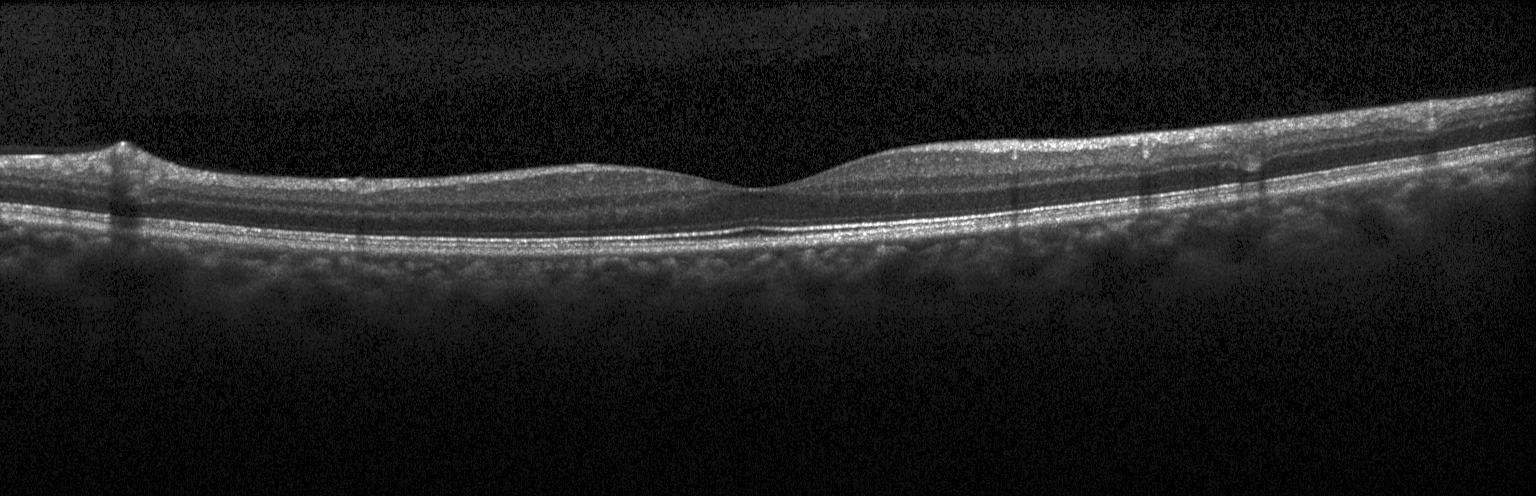

Spectral-domain optical coherence tomography; optical coherence tomography B-scan; fovea-centered; instrument: Heidelberg Spectralis — Impression: neither choroidal neovascularization, diabetic macular edema, nor drusen.